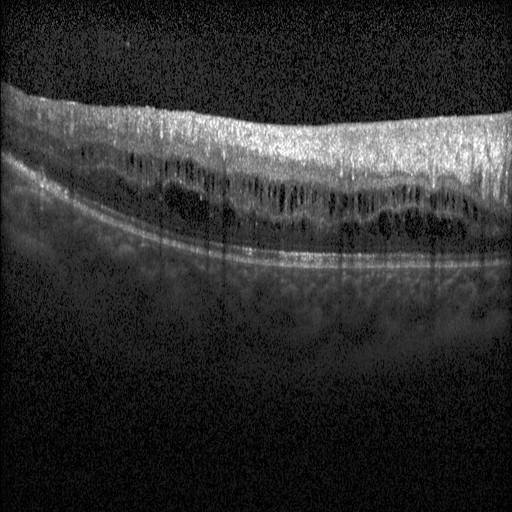 Optical coherence tomography B-scan
Dx: diabetic macular edema.